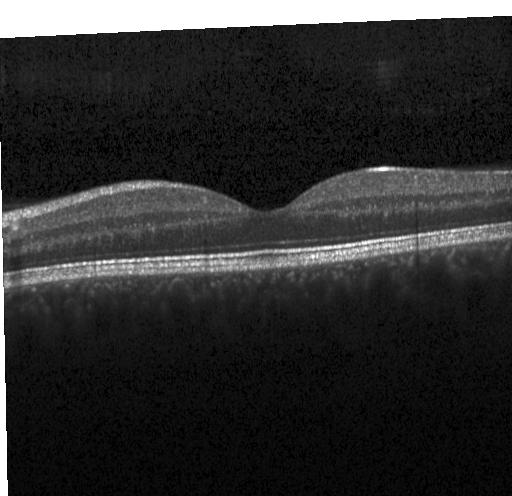

OCT scan showing no choroidal neovascularization, no diabetic macular edema, and no drusen.